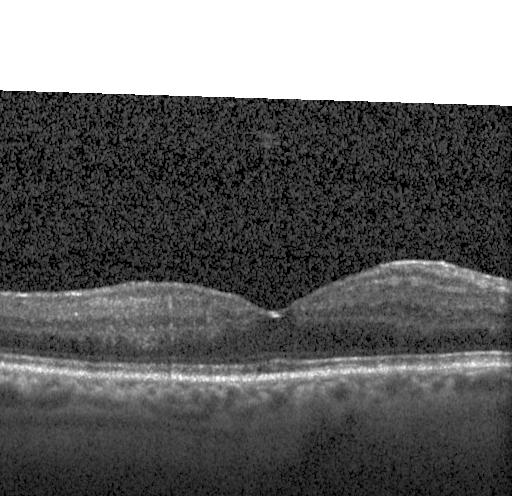
Instrument: Heidelberg Spectralis; retinal OCT cross-section.
OCT finding: neither choroidal neovascularization, diabetic macular edema, nor drusen.